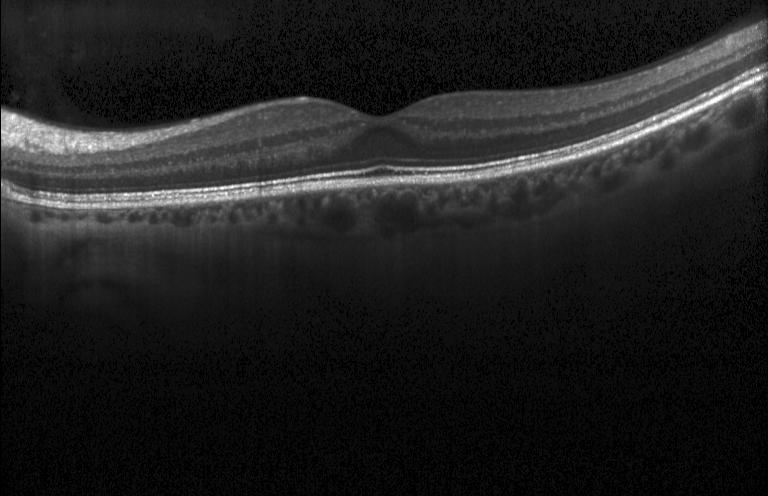

Macular OCT demonstrating no choroidal neovascularization, no diabetic macular edema, and no drusen.